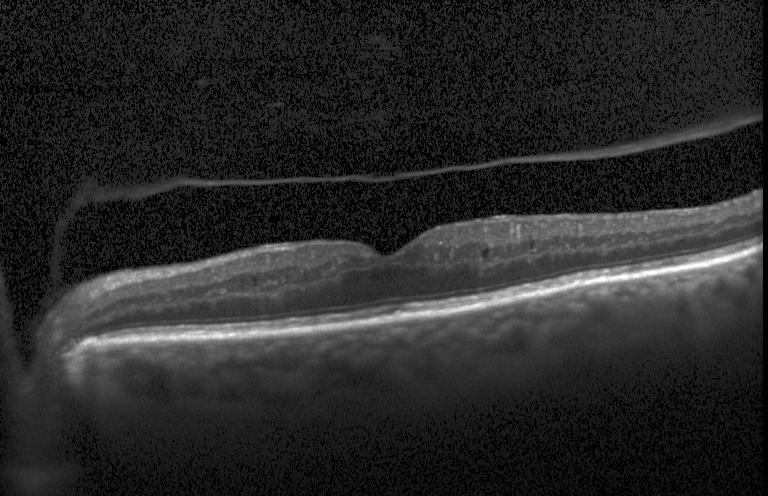 Macular scan, OCT B-scan, spectral-domain OCT — The scan shows DME.